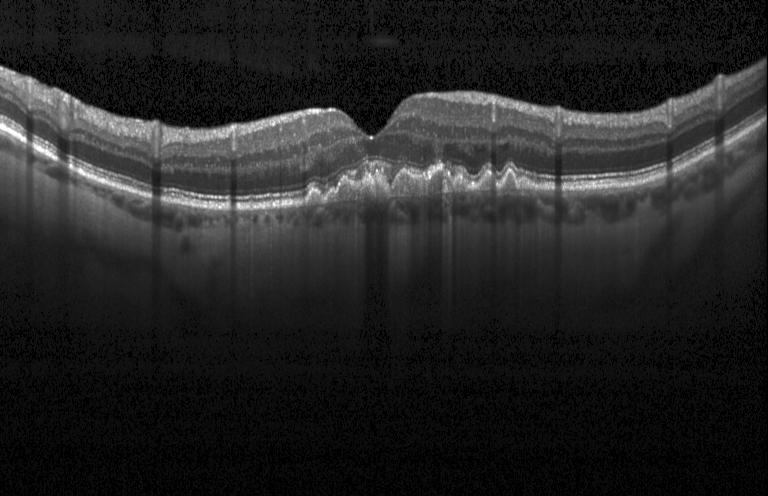
Diagnosis: sub-RPE drusenoid deposits.